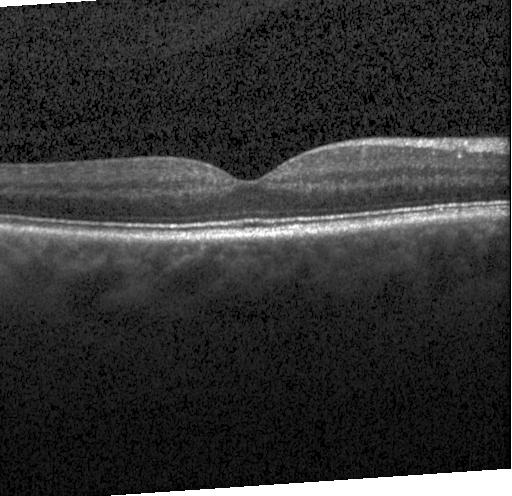 Through the macula; retinal OCT cross-section; SD-OCT; Heidelberg Spectralis OCT system. OCT finding: no choroidal neovascularization, no diabetic macular edema, and no drusen.